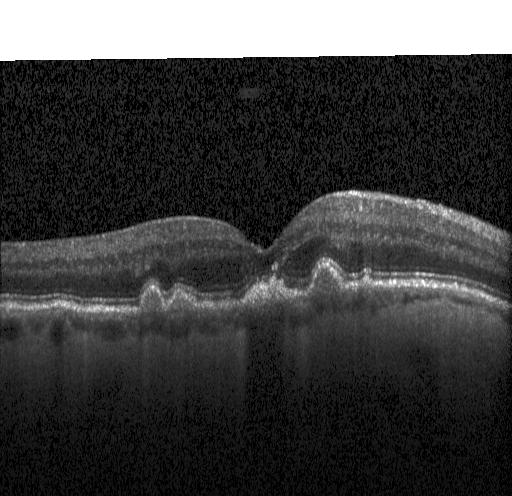

Assessment: multiple drusen.